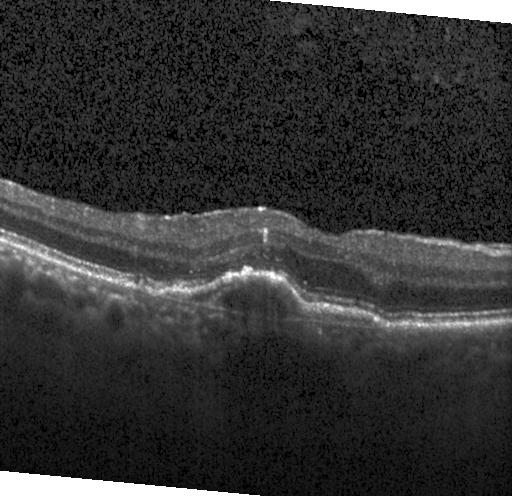

OCT B-scan showing a choroidal neovascular membrane.